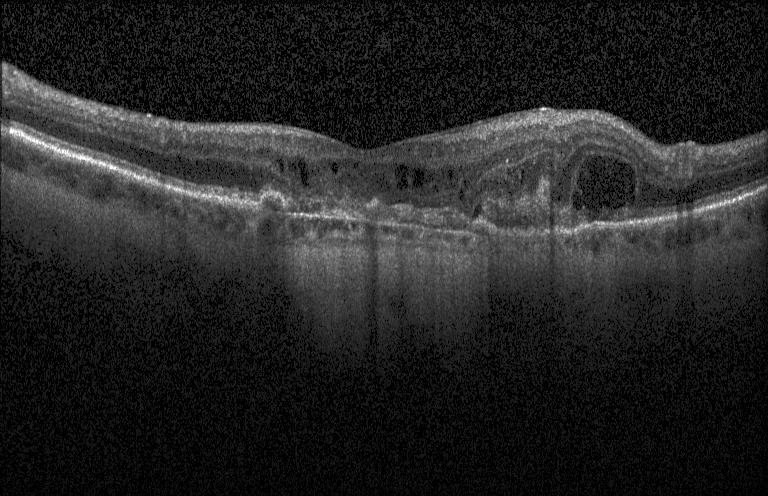

OCT B-scan.
OCT finding: a choroidal neovascular membrane.